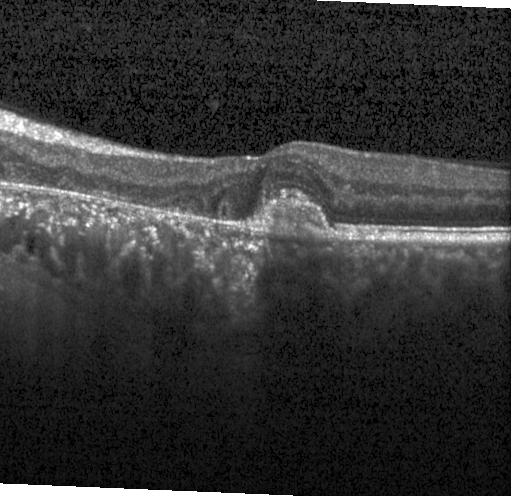 OCT scan showing choroidal neovascularization.